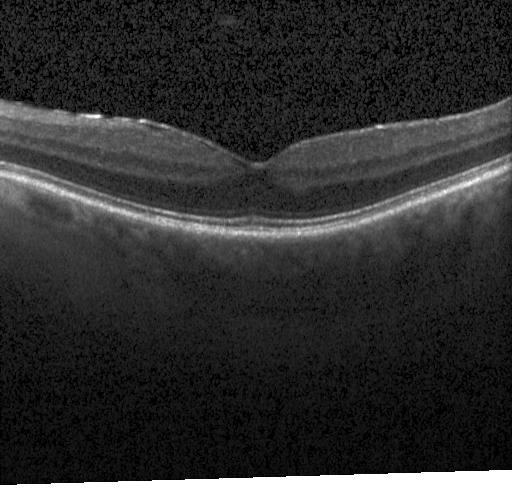
OCT finding: no choroidal neovascularization, no diabetic macular edema, and no drusen.